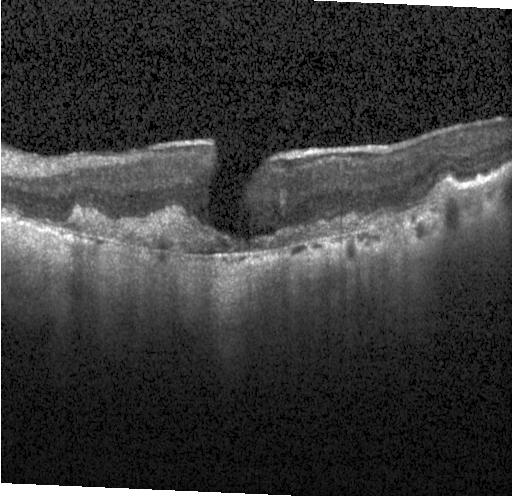
Retinal OCT cross-section · spectral-domain OCT
The scan shows a choroidal neovascular membrane.